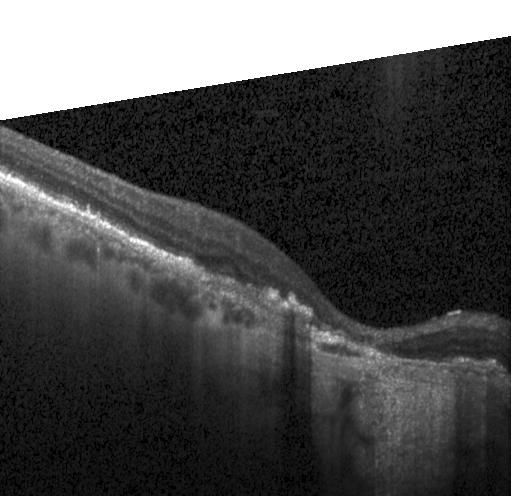
Acquired on a Heidelberg Spectralis · through the macula · retinal OCT B-scan · SD-OCT.
Dx: CNV.